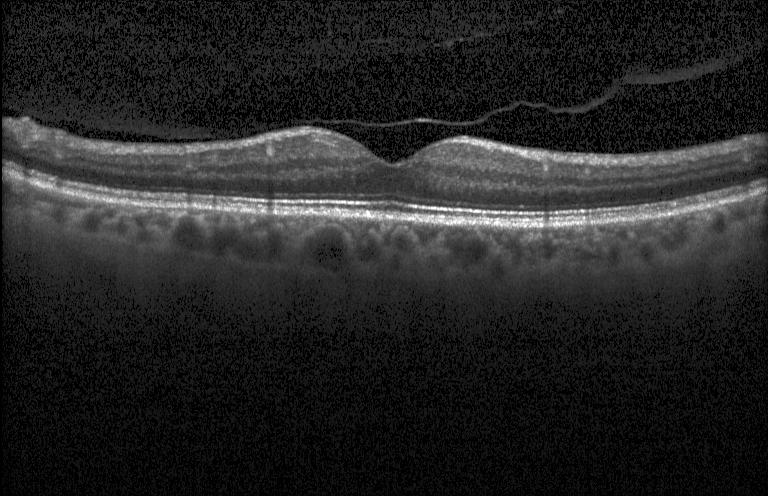

Dx: no evidence of CNV, DME, or drusen.